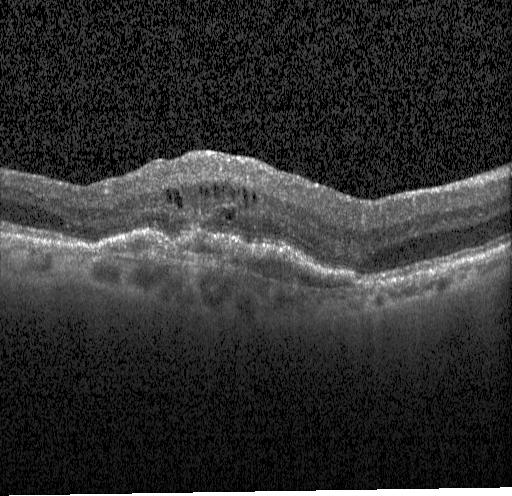

Retinal OCT cross-section.
Impression: choroidal neovascularization.